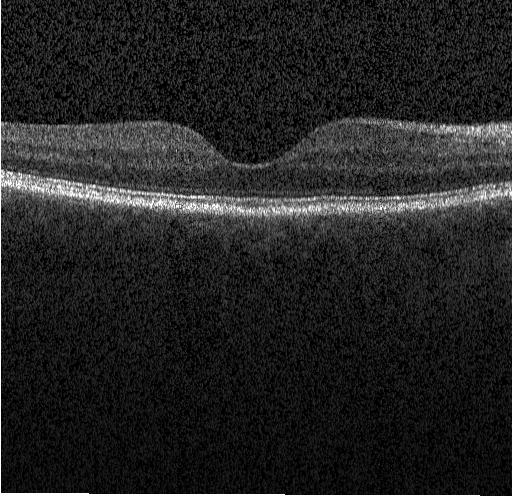

Finding: no choroidal neovascularization, diabetic macular edema, or drusen.